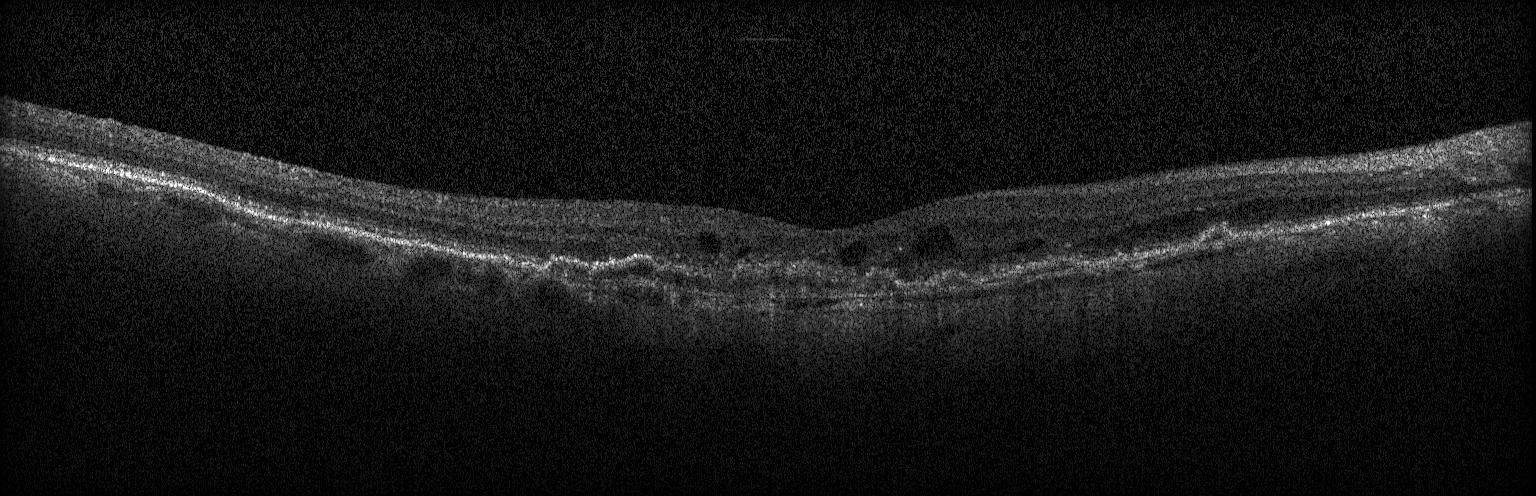

Macular OCT: a choroidal neovascular membrane.